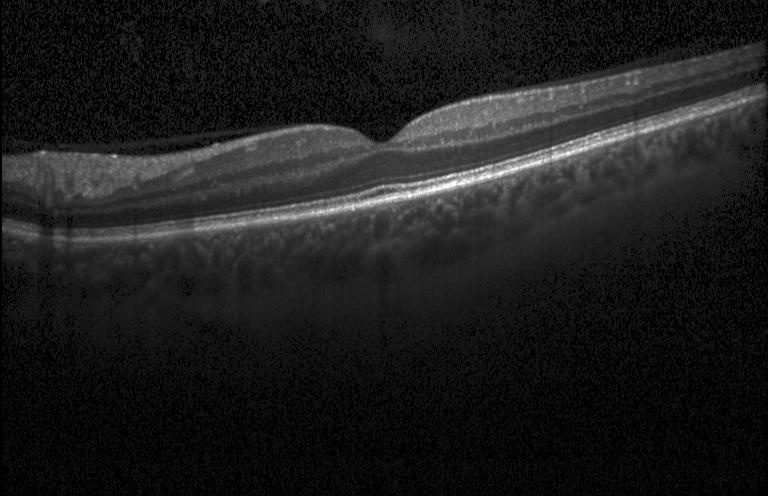
Assessment: neither choroidal neovascularization, diabetic macular edema, nor drusen.